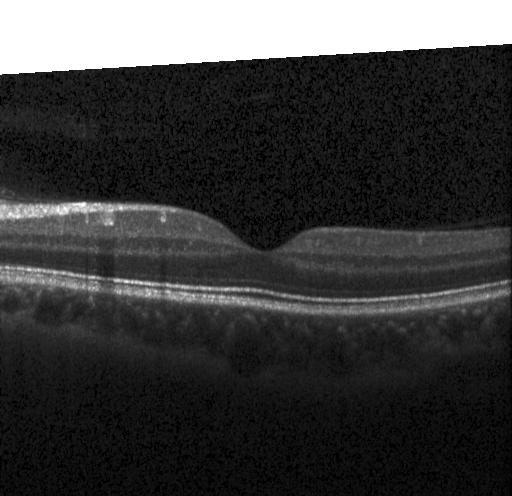 Spectral-domain optical coherence tomography; optical coherence tomography B-scan — Assessment: no choroidal neovascularization, diabetic macular edema, or drusen.